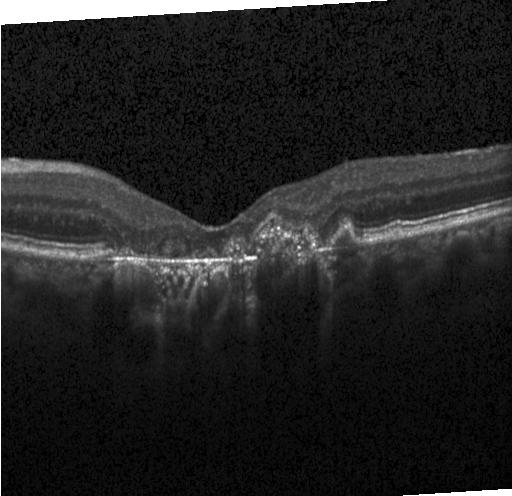

Acquired on a Heidelberg Spectralis · optical coherence tomography B-scan · fovea-centered. Finding: a choroidal neovascular membrane.